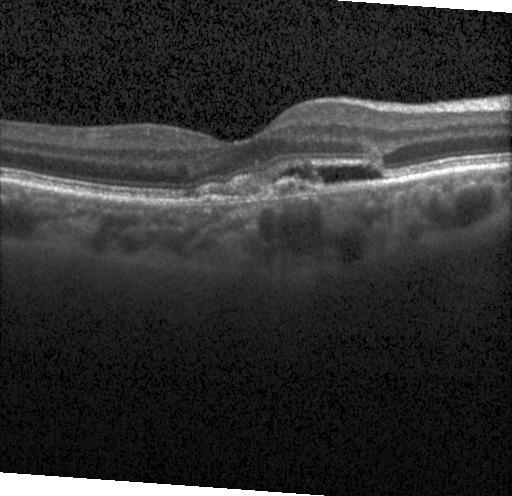 Diagnosis: a choroidal neovascular membrane.